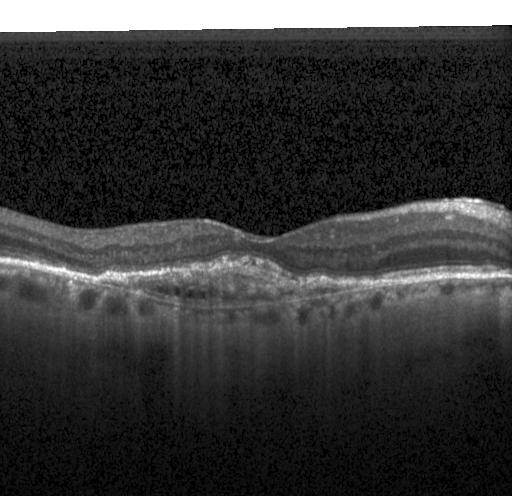 Macular OCT: a choroidal neovascular membrane.